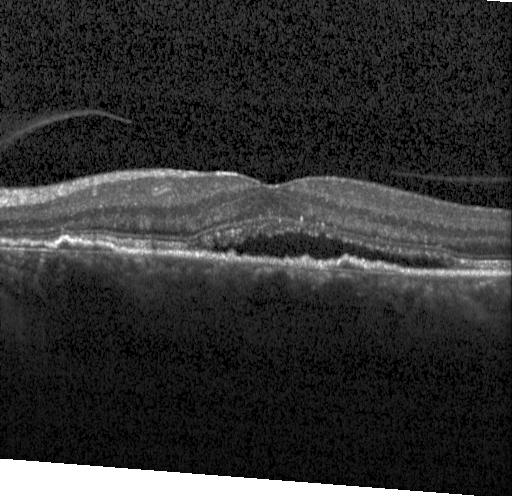
Macular scan; OCT line scan; Heidelberg Spectralis OCT system.
Dx: choroidal neovascularization.